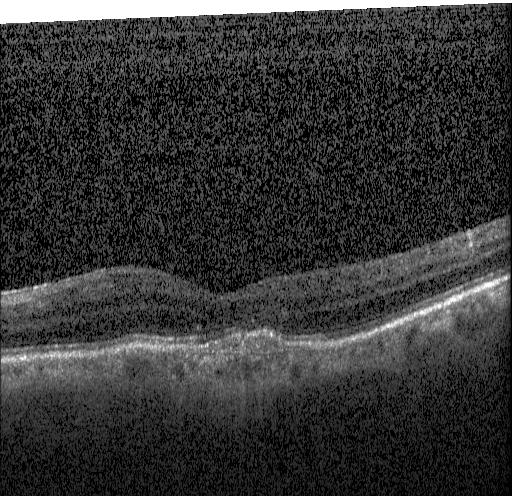
Impression: choroidal neovascularization.